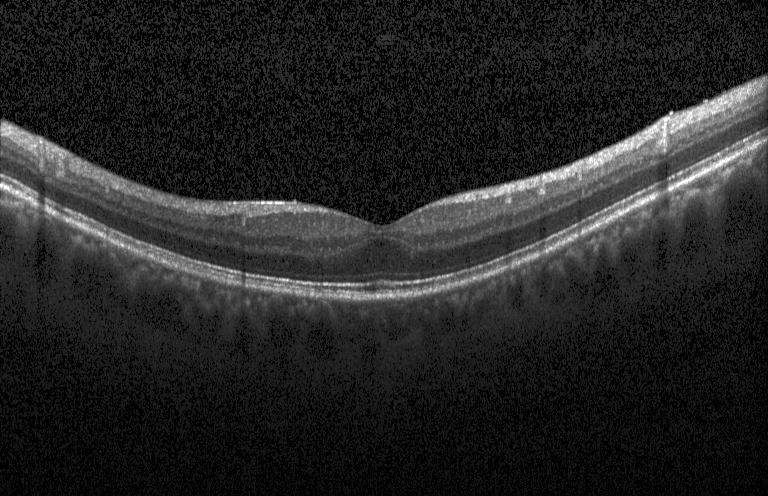
OCT scan showing no CNV, DME, or drusen.